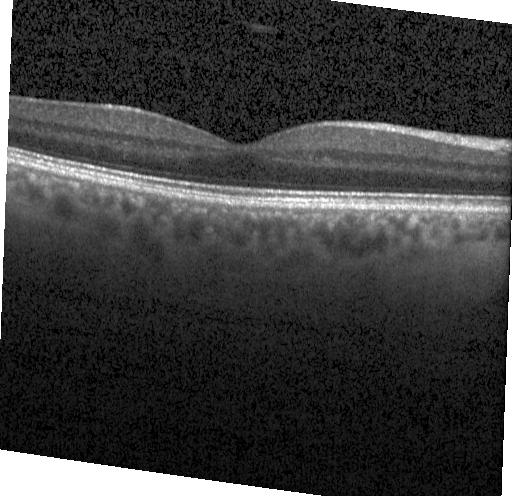

Diagnosis: neither choroidal neovascularization, diabetic macular edema, nor drusen.